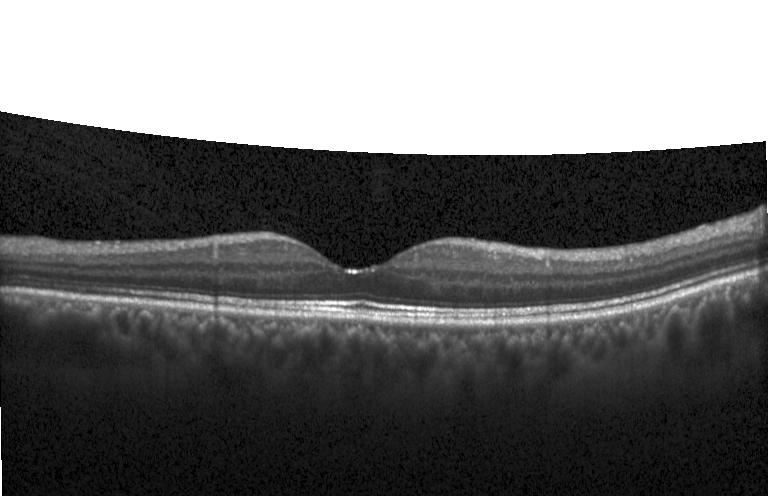

Spectral-domain optical coherence tomography. Optical coherence tomography B-scan. Macular scan.
Assessment: no evidence of CNV, DME, or drusen.